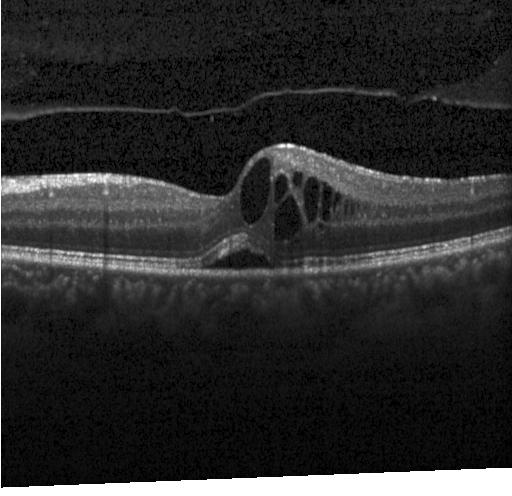 Assessment: diabetic macular edema (DME).